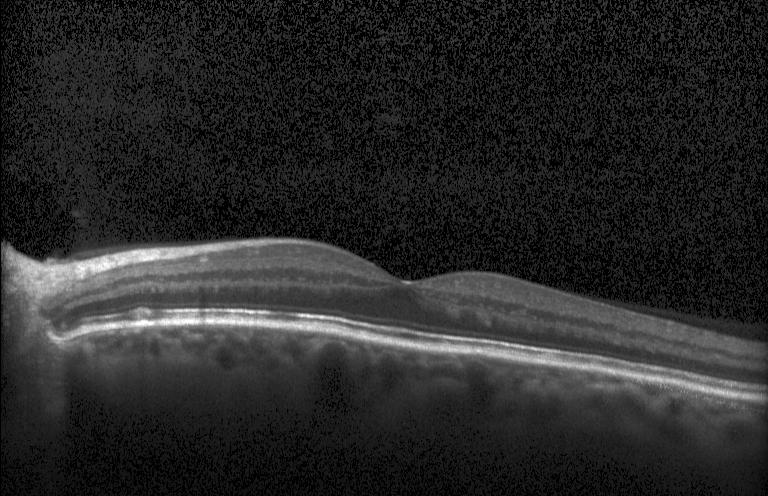

OCT B-scan showing neither CNV, DME, nor drusen.